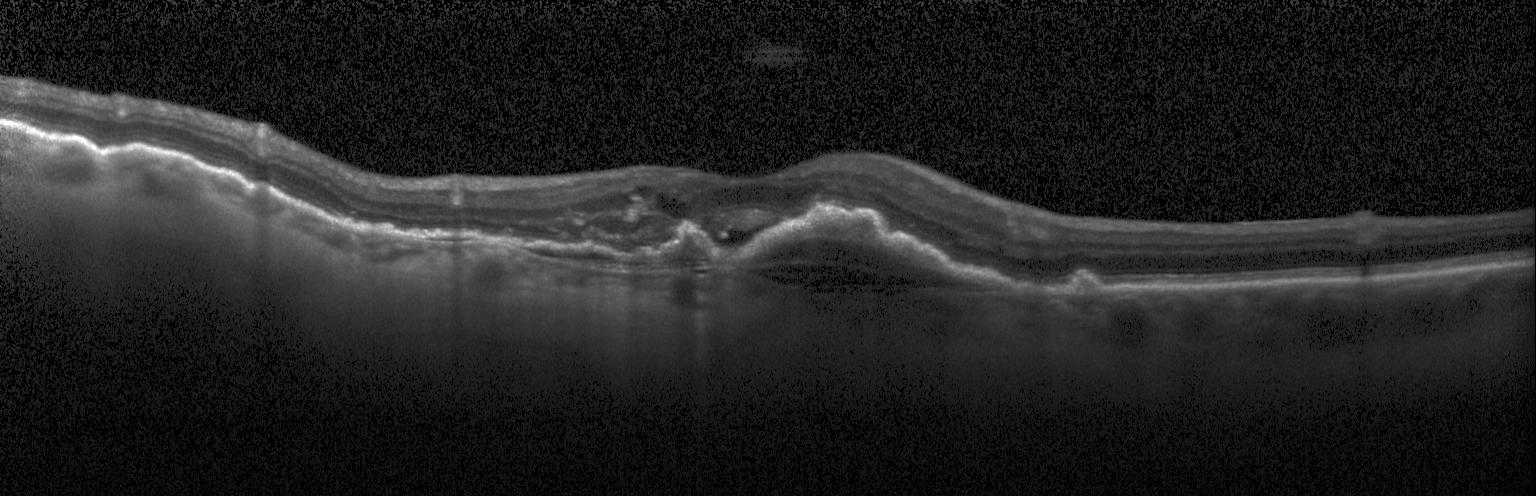 OCT finding: a choroidal neovascular membrane.